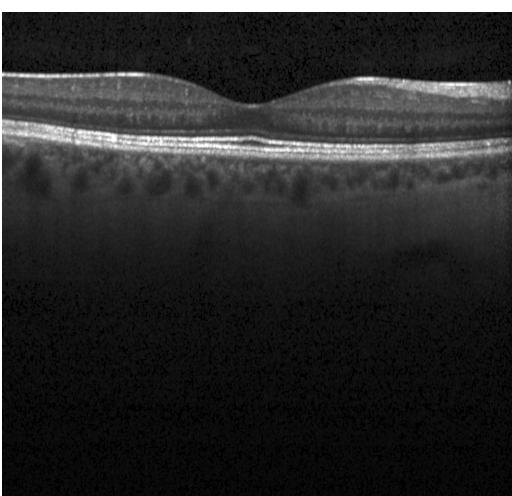 Retinal OCT B-scan, macular scan, acquired on a Heidelberg Spectralis — Assessment: neither choroidal neovascularization, diabetic macular edema, nor drusen.